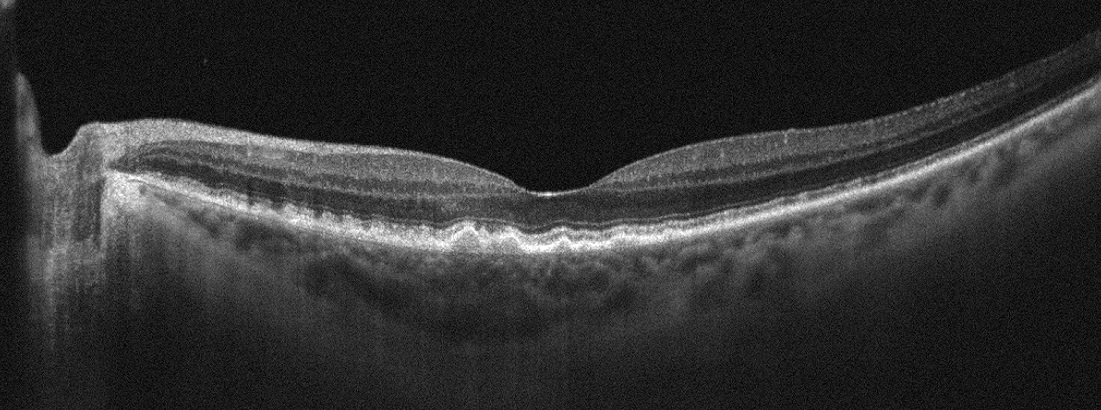 OCT B-scan. Impression: age-related macular degeneration (AMD).